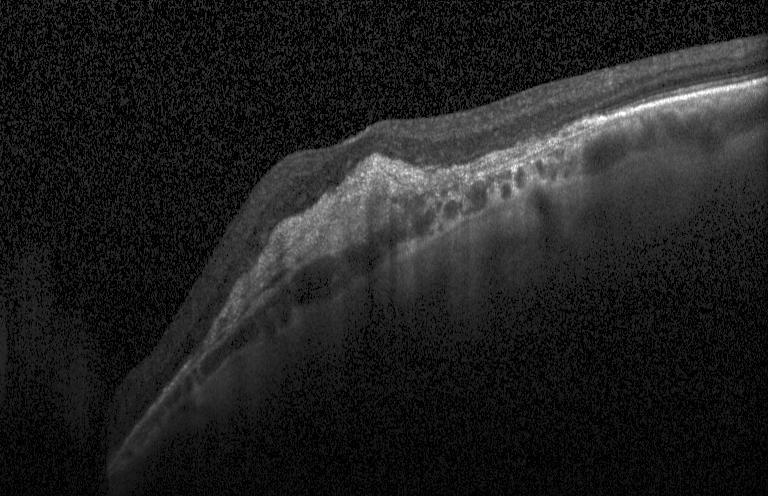 Through the macula; SD-OCT; retinal OCT B-scan — Diagnosis: choroidal neovascularization.